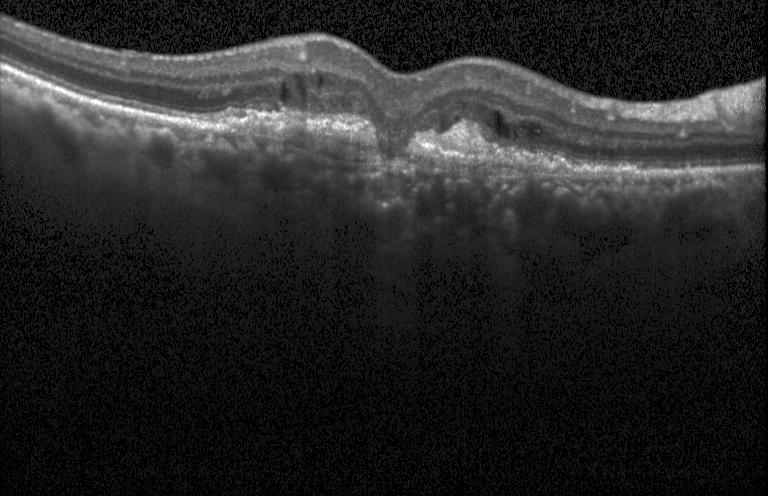

OCT line scan; Heidelberg Spectralis; horizontal scan through the fovea; spectral-domain optical coherence tomography
Finding: choroidal neovascularization (CNV).